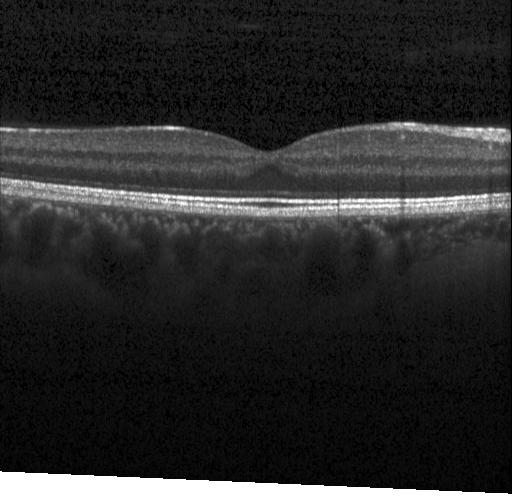 Fovea-centered · OCT B-scan — Macular OCT: no choroidal neovascularization, diabetic macular edema, or drusen.